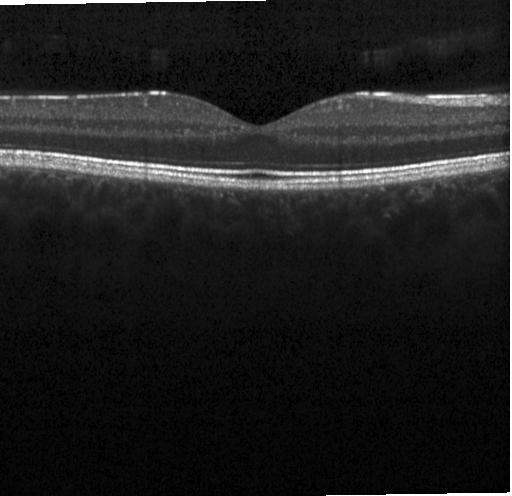
Spectral-domain optical coherence tomography · instrument: Heidelberg Spectralis · OCT line scan · fovea-centered
The scan shows no choroidal neovascularization, no diabetic macular edema, and no drusen.